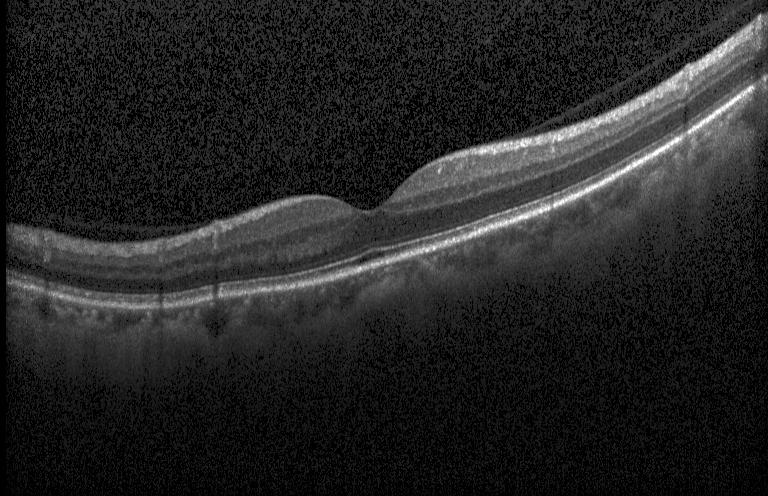

Impression: no evidence of choroidal neovascularization, diabetic macular edema, or drusen.